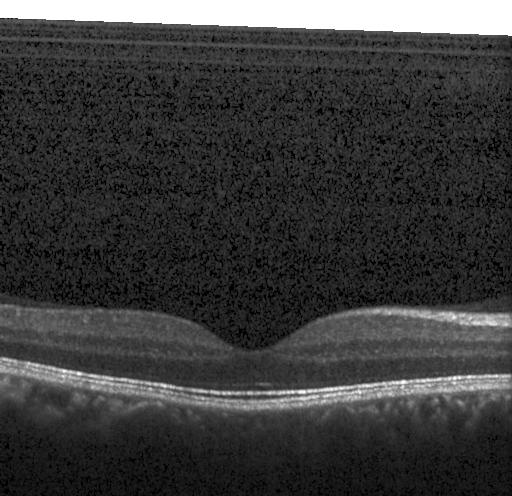
Retinal OCT B-scan
Finding: no evidence of choroidal neovascularization, diabetic macular edema, or drusen.